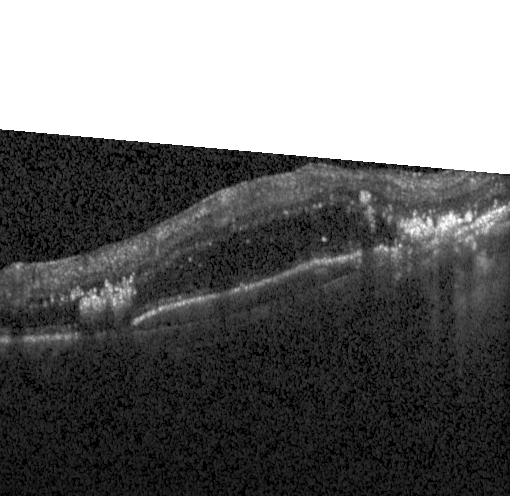

The scan shows DME.